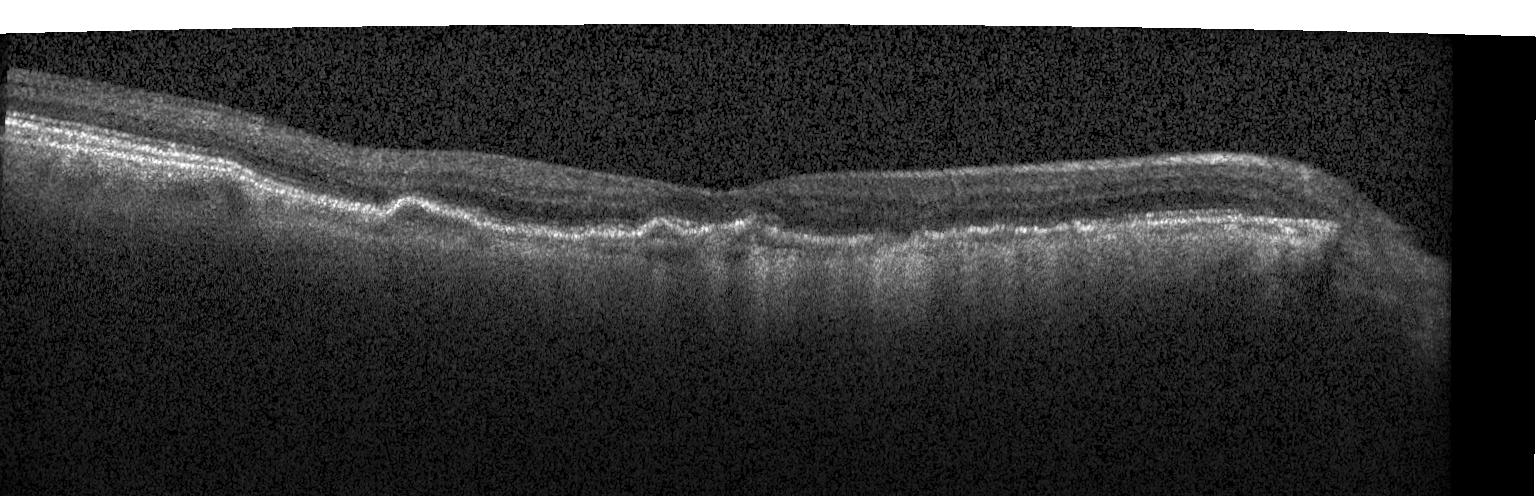

Retinal OCT cross-section. Centered on the fovea. SD-OCT. Acquired on a Heidelberg Spectralis. Dx: choroidal neovascularization (CNV).